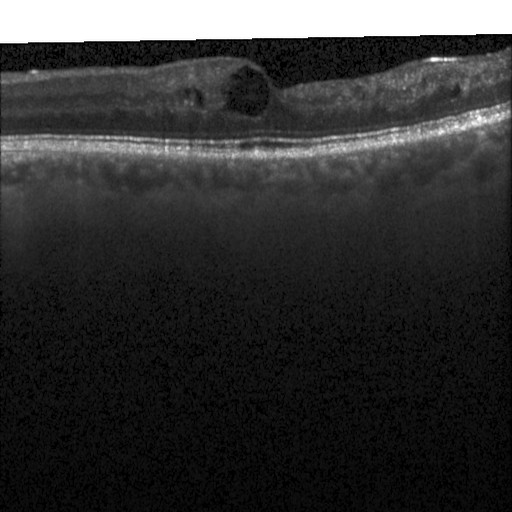
Finding: diabetic macular edema.